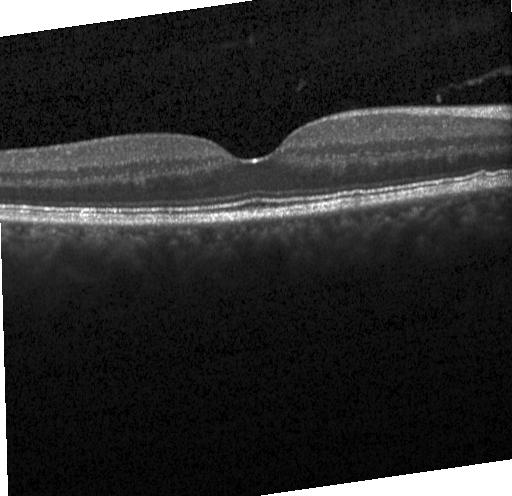

OCT B-scan — Diagnosis: no choroidal neovascularization, no diabetic macular edema, and no drusen.